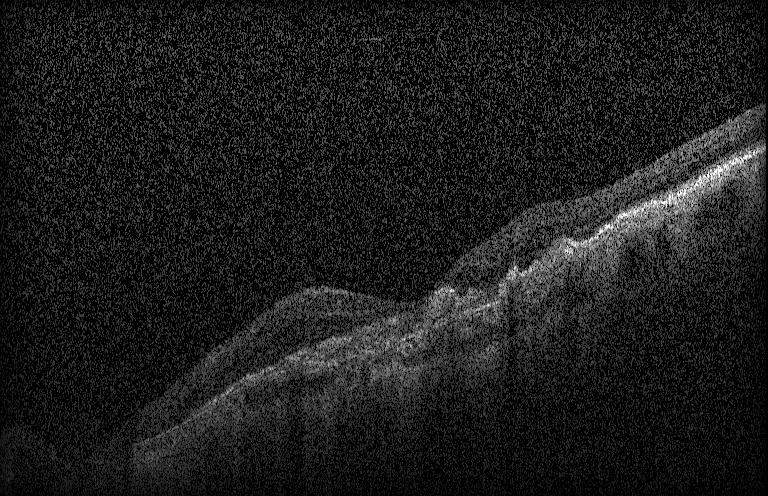 Retinal OCT B-scan — Finding: a choroidal neovascular membrane.